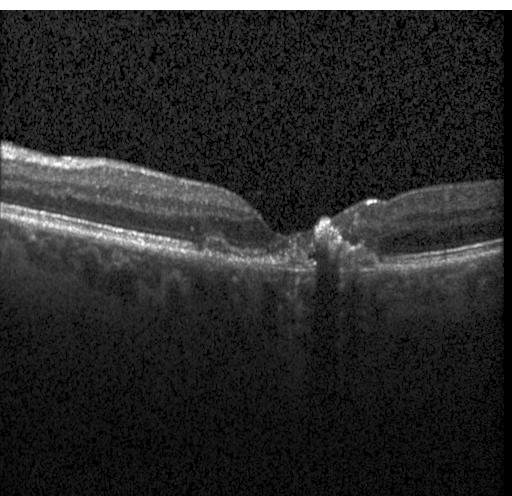
OCT B-scan, Heidelberg Spectralis — Finding: CNV.